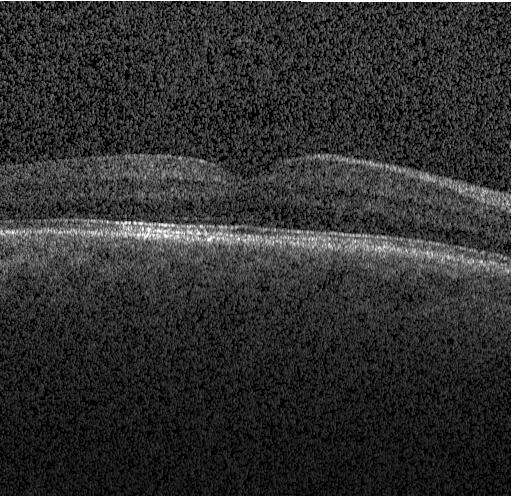
OCT B-scan
OCT finding: no evidence of choroidal neovascularization, diabetic macular edema, or drusen.